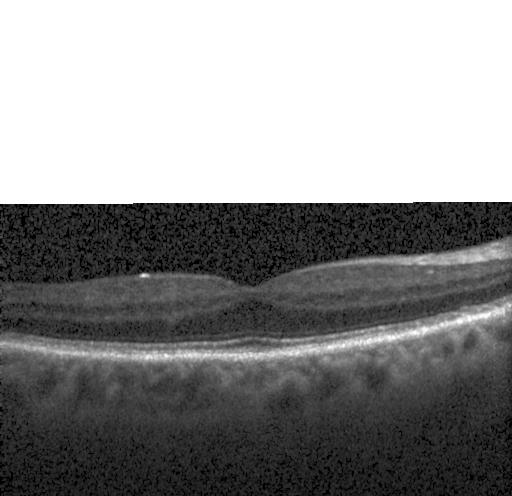

Through the macula · spectral-domain optical coherence tomography · OCT line scan — Assessment: no evidence of CNV, DME, or drusen.